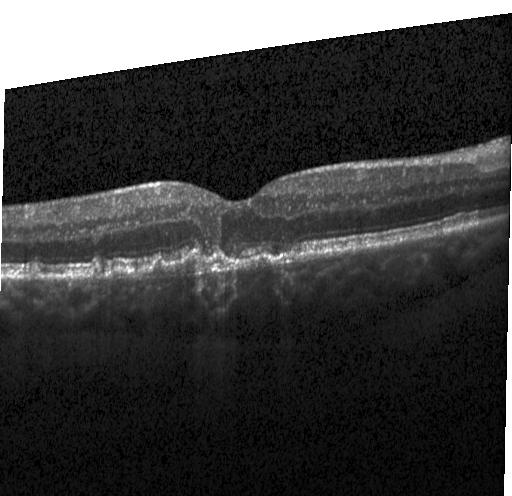
OCT B-scan · instrument: Heidelberg Spectralis. The scan shows choroidal neovascularization (CNV).